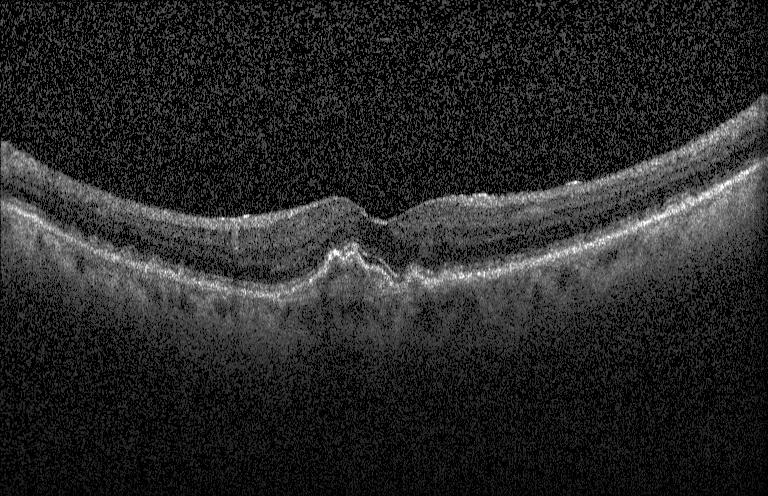

OCT scan showing choroidal neovascularization.